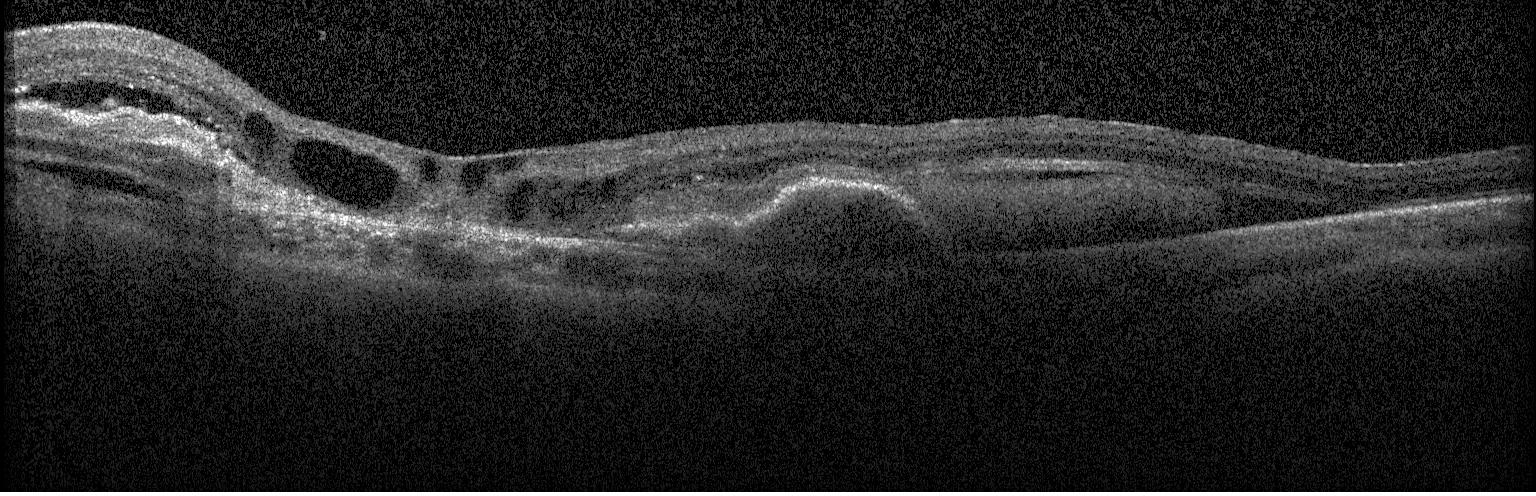

Retinal OCT B-scan. Fovea-centered. SD-OCT. Acquired on a Heidelberg Spectralis
Impression: a choroidal neovascular membrane.